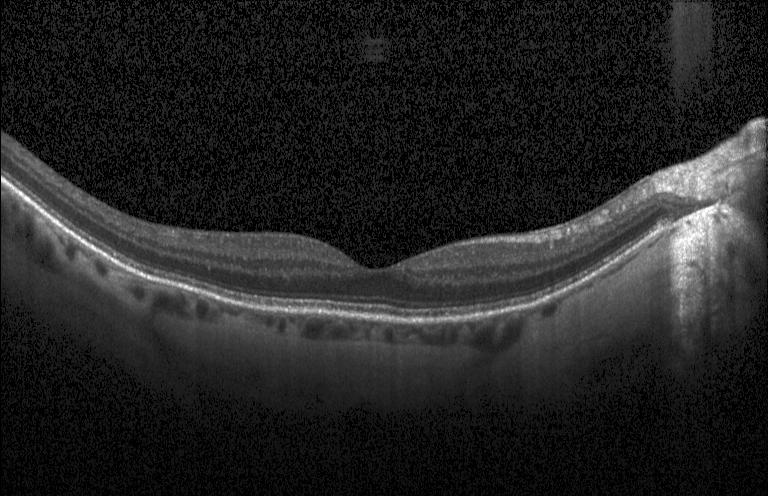
Heidelberg Spectralis OCT system. OCT line scan. Macular scan.
The scan shows no choroidal neovascularization, no diabetic macular edema, and no drusen.